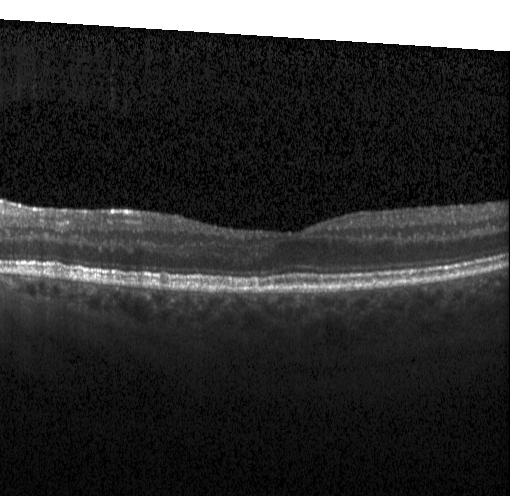

Centered on the fovea, optical coherence tomography B-scan, Heidelberg Spectralis — Finding: no CNV, DME, or drusen.